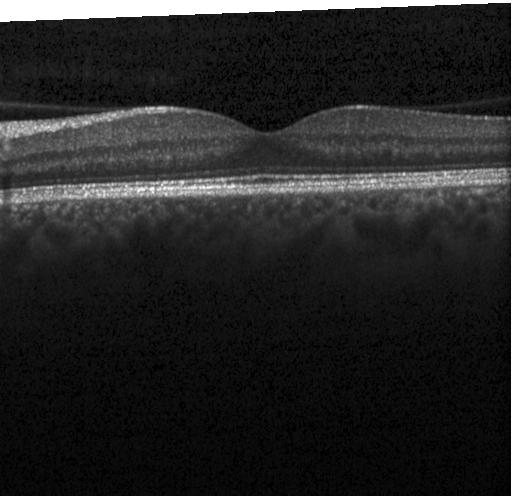
Spectral-domain OCT; through the macula; optical coherence tomography B-scan.
This B-scan demonstrates neither choroidal neovascularization, diabetic macular edema, nor drusen.